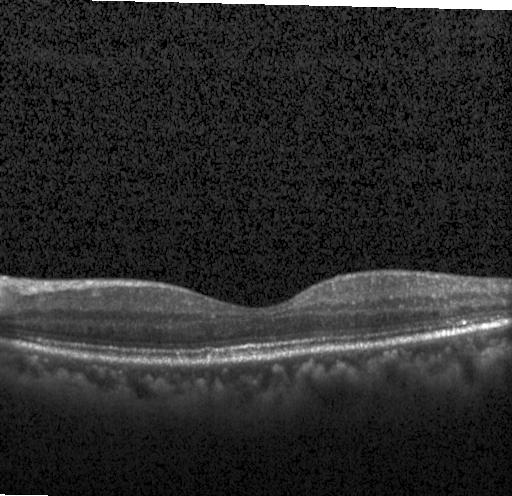

No CNV, no DME, and no drusen.